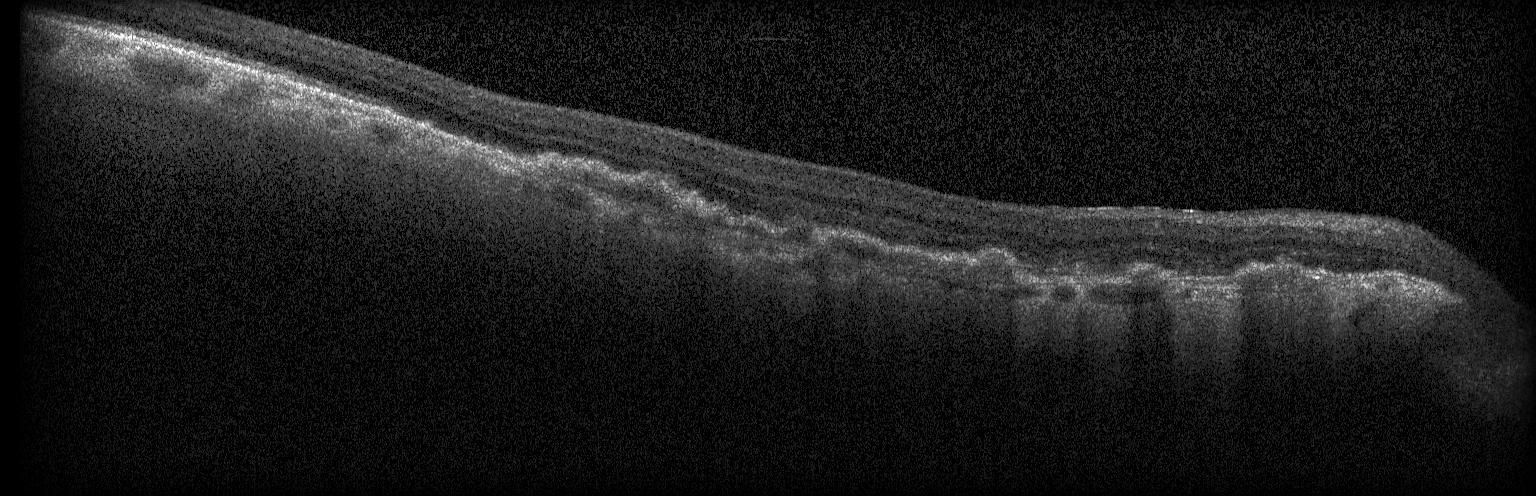

Retinal OCT cross-section. SD-OCT. Heidelberg Spectralis OCT system. Dx: a choroidal neovascular membrane.